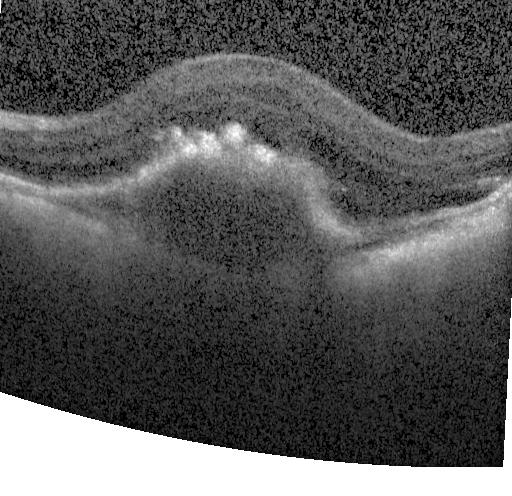

This B-scan demonstrates choroidal neovascularization (CNV).